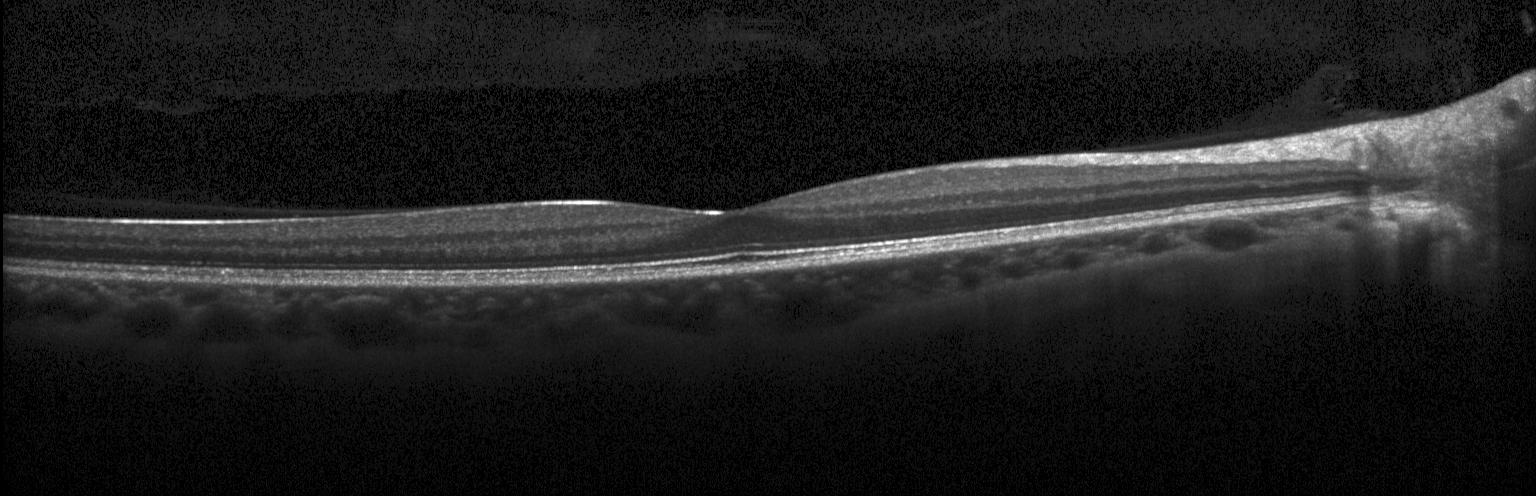 Dx: neither choroidal neovascularization, diabetic macular edema, nor drusen.